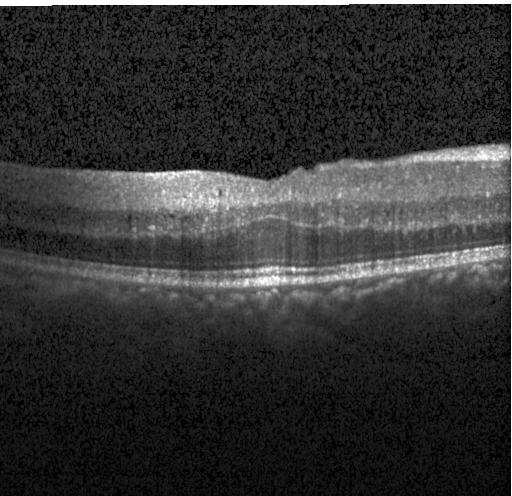

Retinal OCT cross-section; fovea-centered; SD-OCT. Diabetic macular edema (DME).